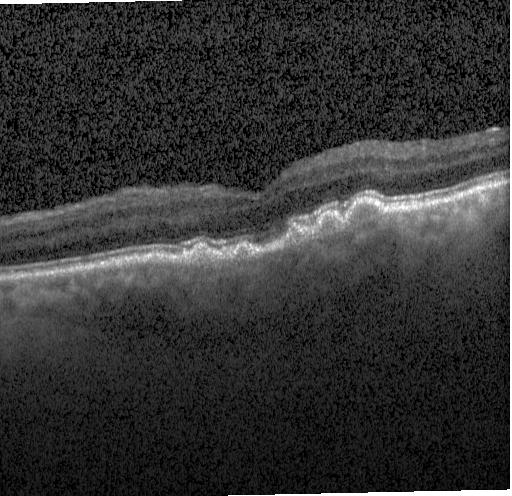

Finding: drusen.